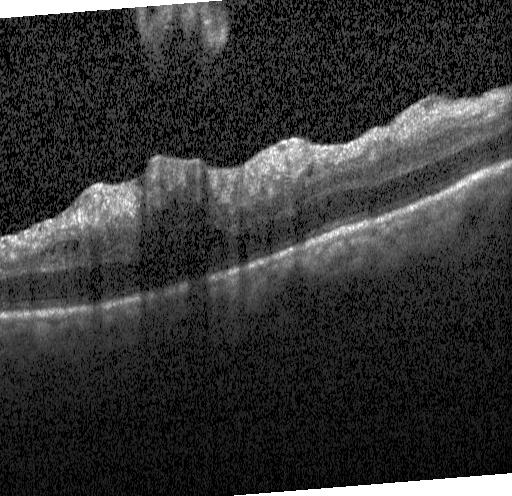
Dx: DME.